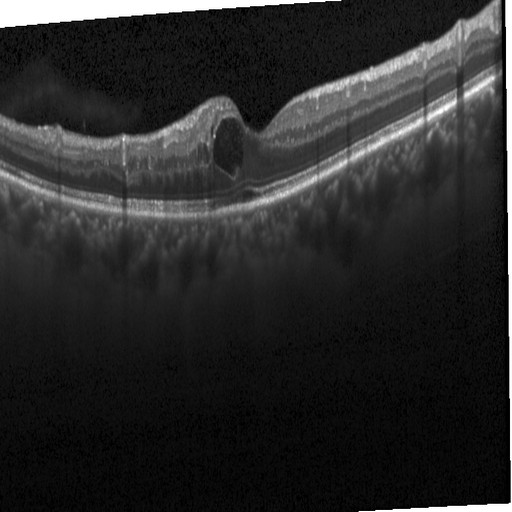
Retinal OCT cross-section — Assessment: diabetic macular edema (DME).